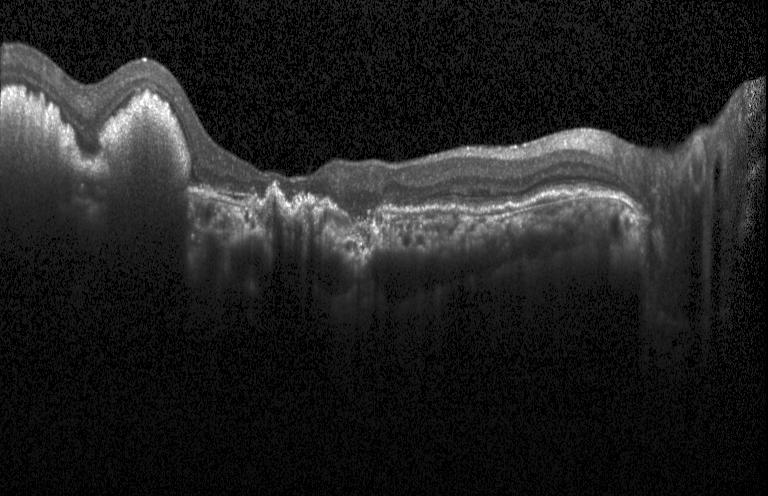 Macular scan. SD-OCT. Retinal OCT cross-section.
The scan shows a choroidal neovascular membrane.